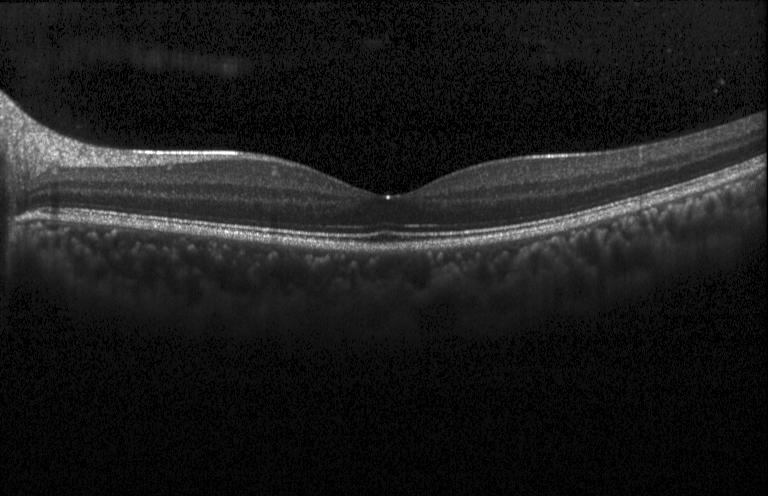 Spectral-domain OCT. Retinal OCT B-scan. Instrument: Heidelberg Spectralis. Horizontal scan through the fovea
Macular OCT: neither CNV, DME, nor drusen.